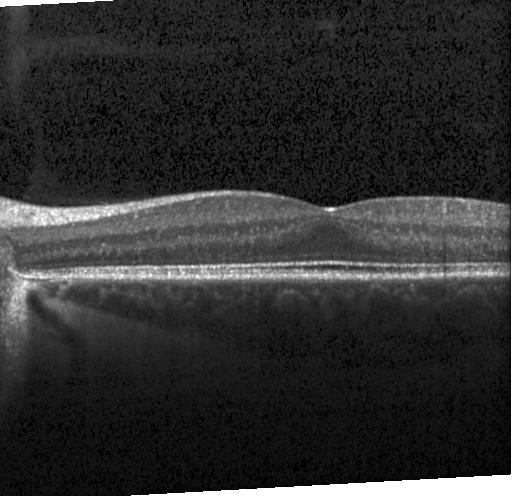 Optical coherence tomography B-scan — Impression: no evidence of CNV, DME, or drusen.